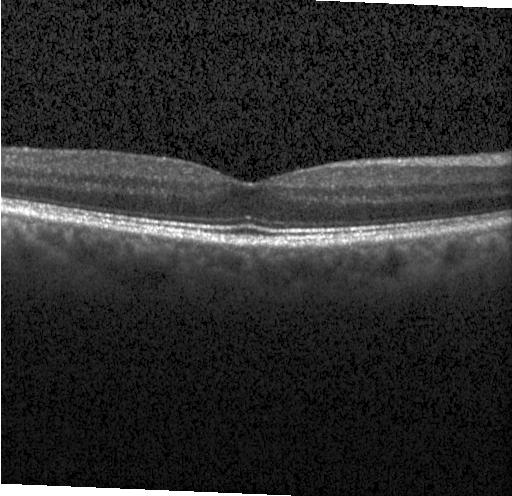

This B-scan demonstrates no choroidal neovascularization, diabetic macular edema, or drusen.